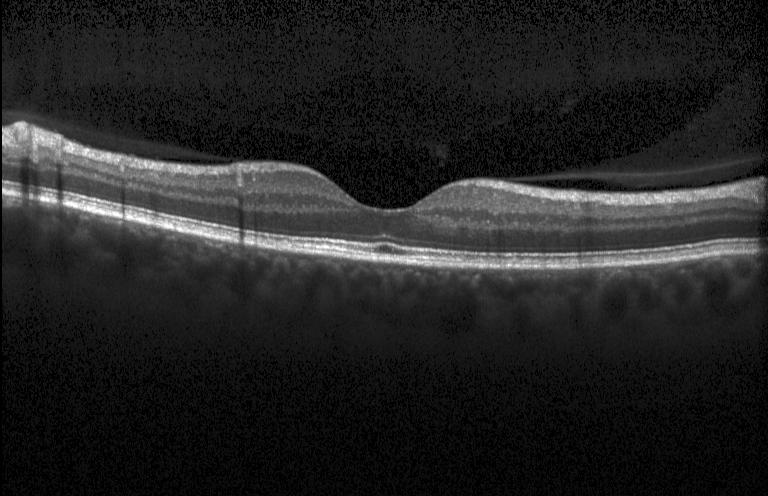

OCT B-scan showing no CNV, no DME, and no drusen.